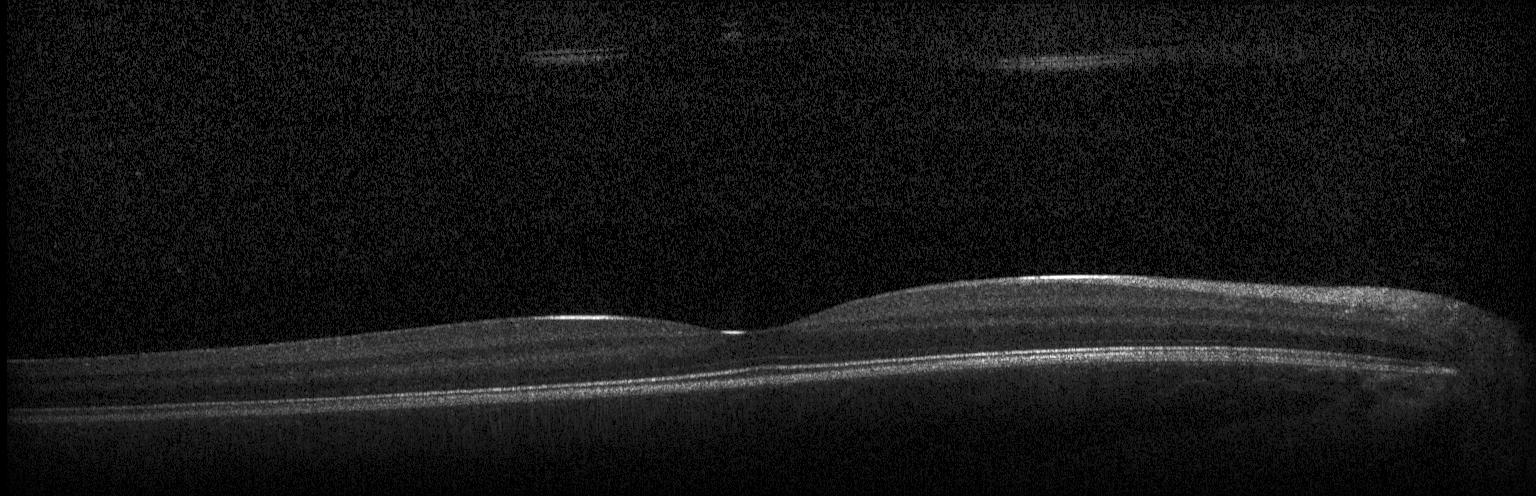
Spectral-domain OCT. Retinal OCT cross-section
Assessment: no evidence of CNV, DME, or drusen.